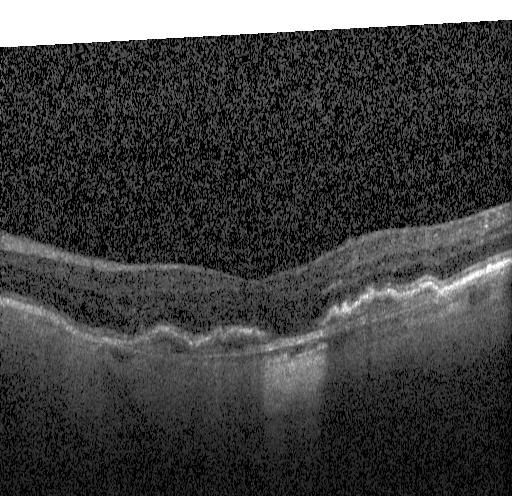 Centered on the fovea · SD-OCT · OCT B-scan. Diagnosis: a choroidal neovascular membrane.